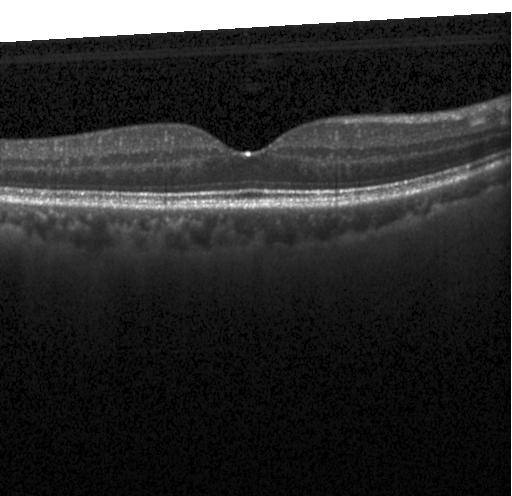

Retinal OCT B-scan
Finding: no CNV, DME, or drusen.